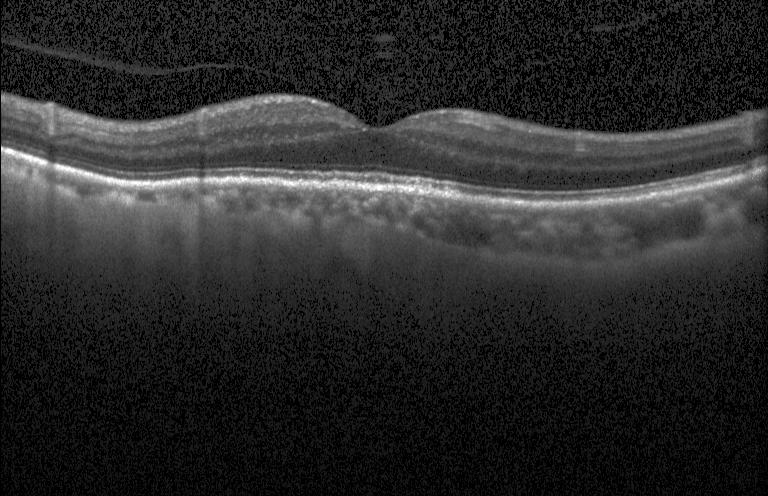
SD-OCT, retinal OCT B-scan, fovea-centered, Heidelberg Spectralis OCT system.
Assessment: no evidence of CNV, DME, or drusen.